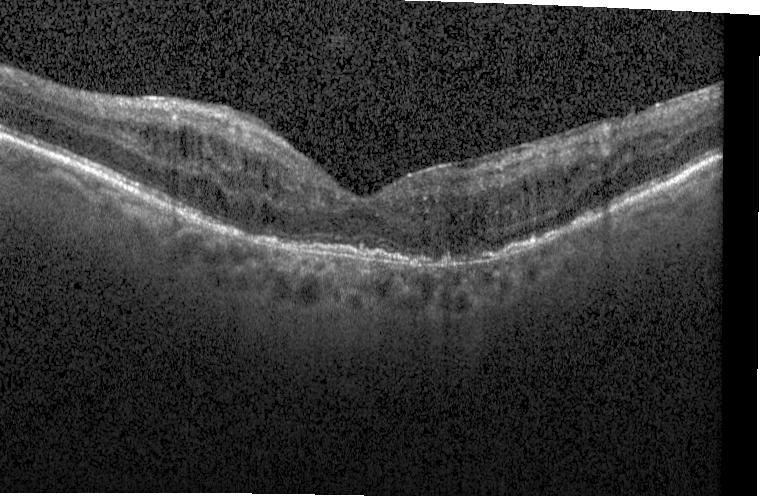
Optical coherence tomography B-scan — The scan shows choroidal neovascularization.